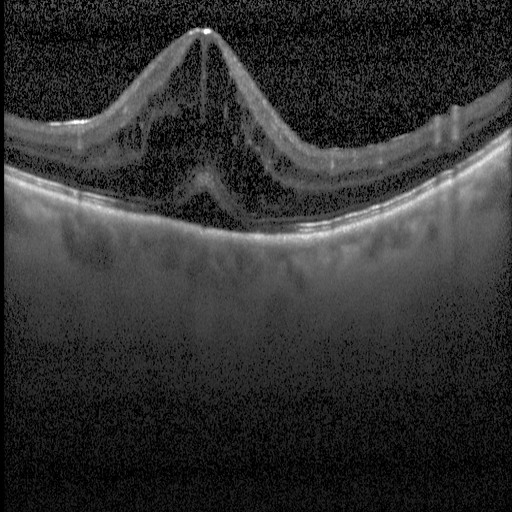
Optical coherence tomography B-scan — Assessment: diabetic macular edema (DME).